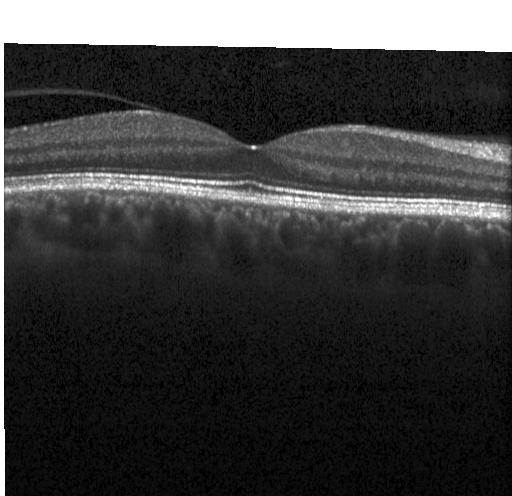
Spectral-domain OCT, macular scan, OCT line scan. This B-scan demonstrates no choroidal neovascularization, no diabetic macular edema, and no drusen.